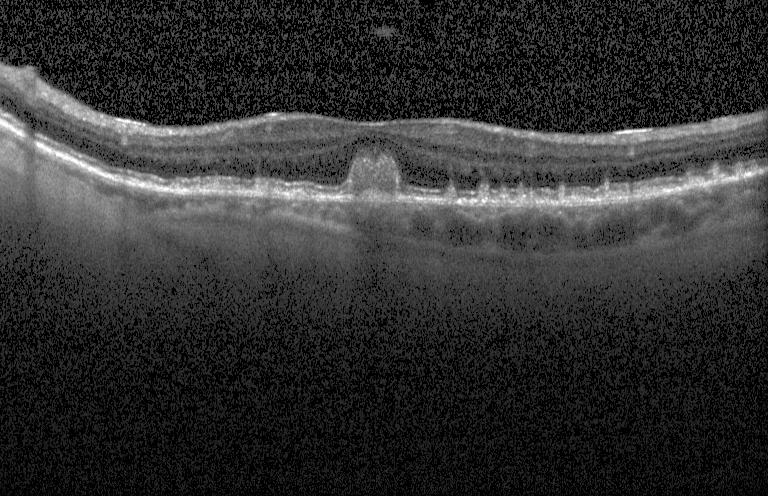 Horizontal scan through the fovea; Heidelberg Spectralis; OCT B-scan.
Assessment: CNV.